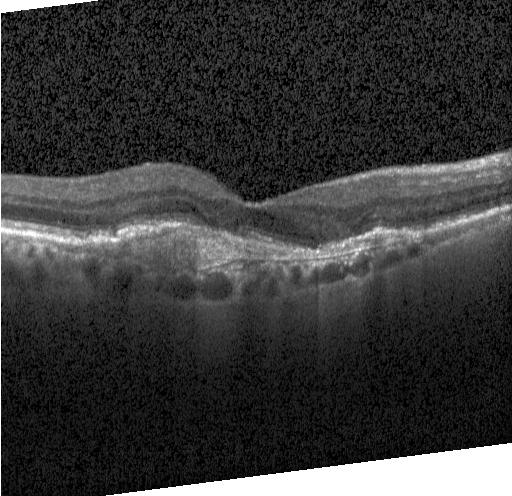
Spectral-domain OCT · optical coherence tomography scan.
Diagnosis: a choroidal neovascular membrane.